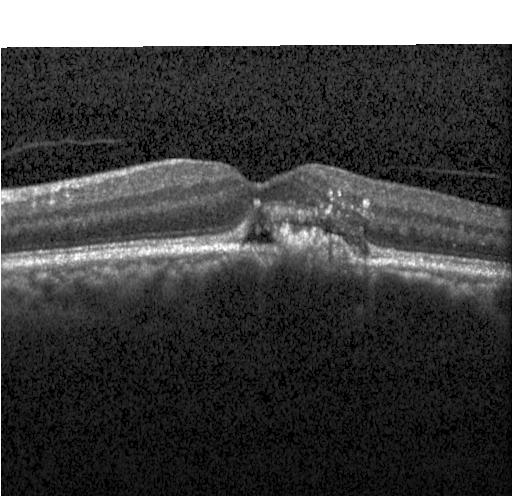 A choroidal neovascular membrane.